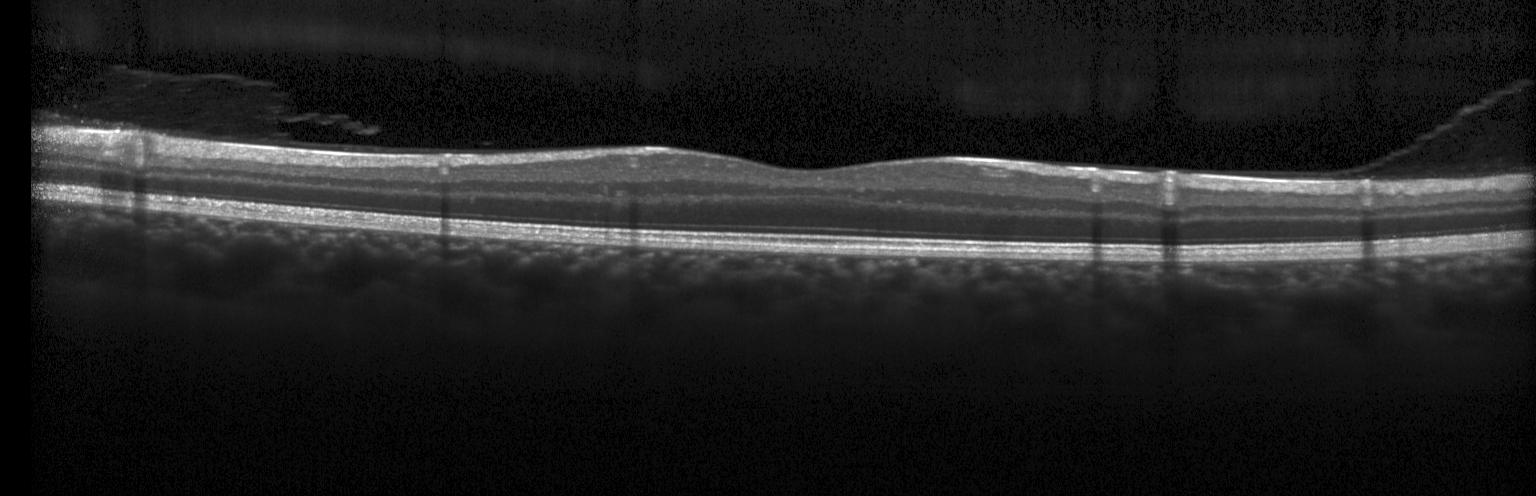 Heidelberg Spectralis. Macular scan. OCT B-scan
This B-scan demonstrates no evidence of CNV, DME, or drusen.